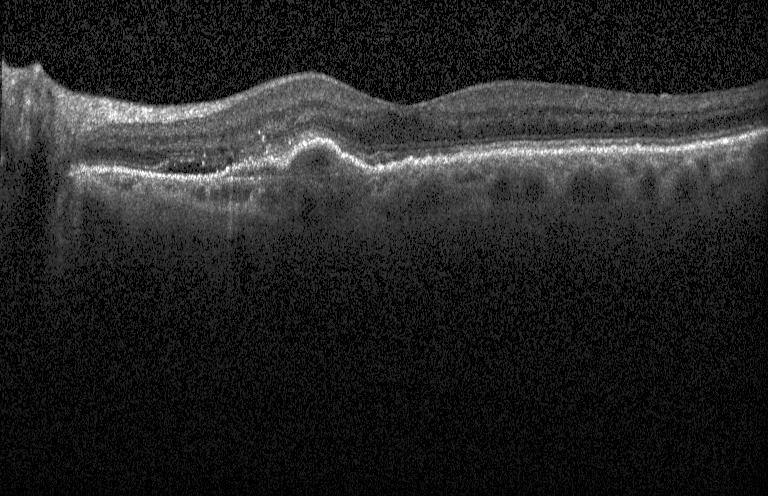

Optical coherence tomography scan; through the macula; acquired on a Heidelberg Spectralis; spectral-domain optical coherence tomography.
Diagnosis: a choroidal neovascular membrane.